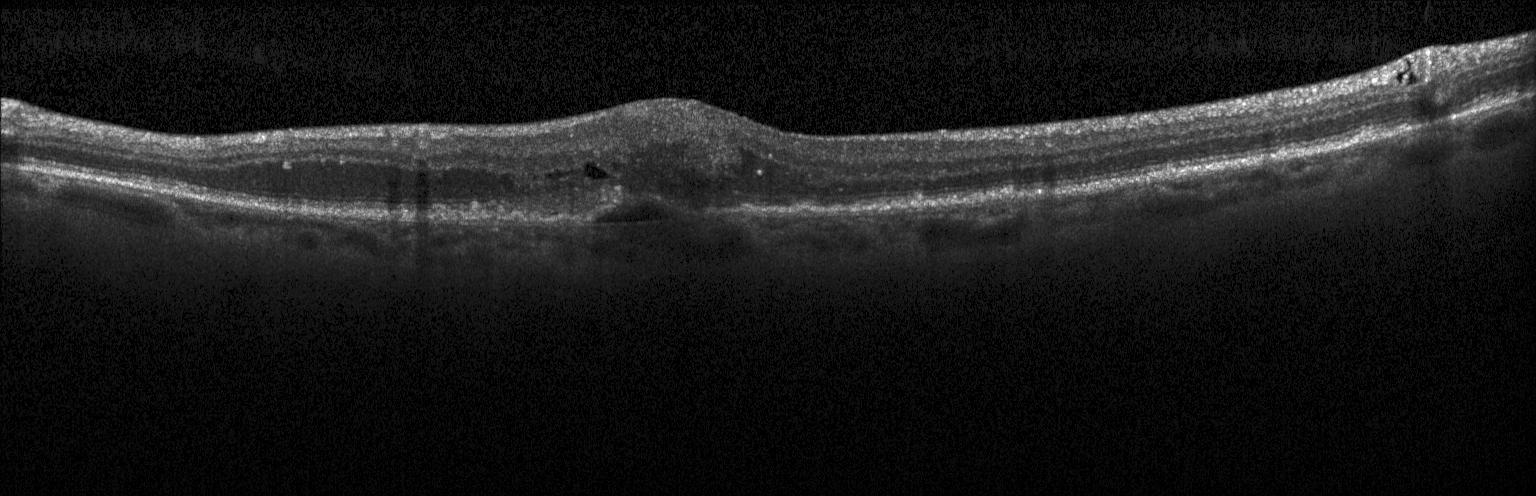

OCT scan showing CNV.